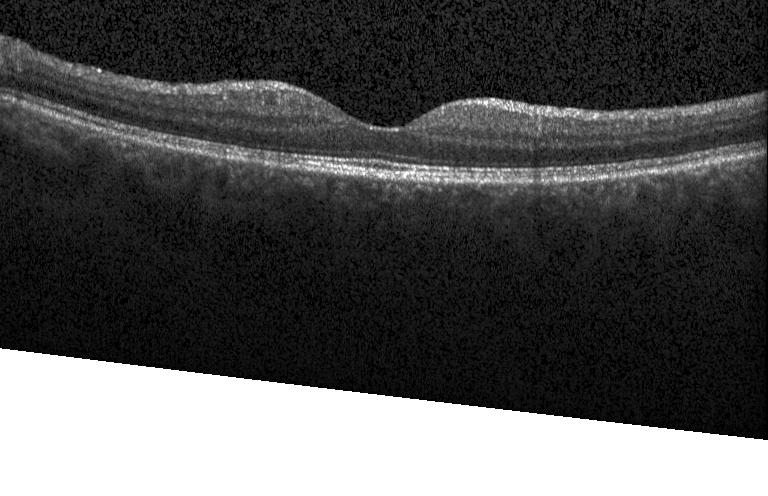 OCT line scan · spectral-domain optical coherence tomography · instrument: Heidelberg Spectralis — OCT finding: neither CNV, DME, nor drusen.